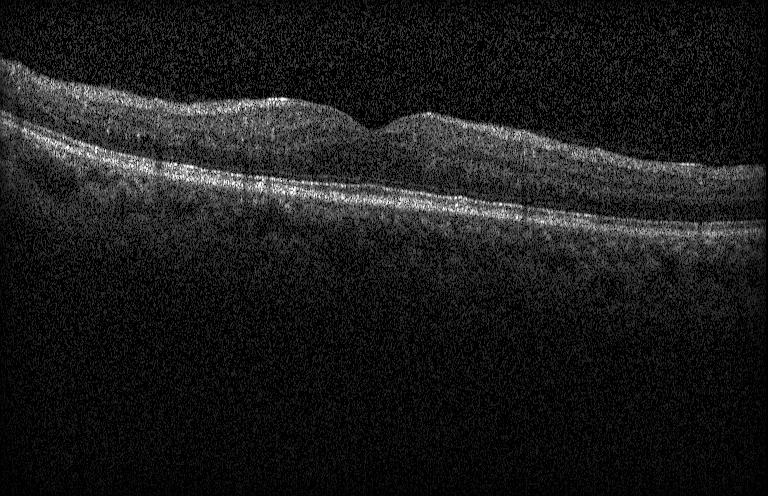 Retinal OCT B-scan. Macular scan. SD-OCT — OCT finding: no choroidal neovascularization, no diabetic macular edema, and no drusen.